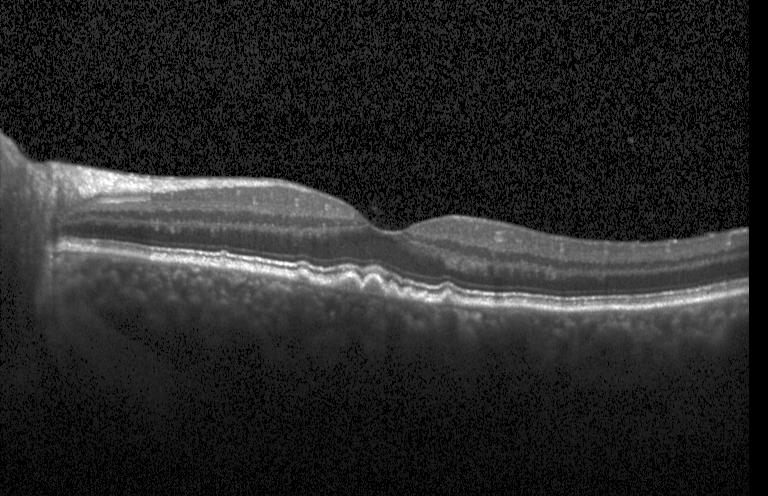 Retinal OCT cross-section. The scan shows multiple drusen.